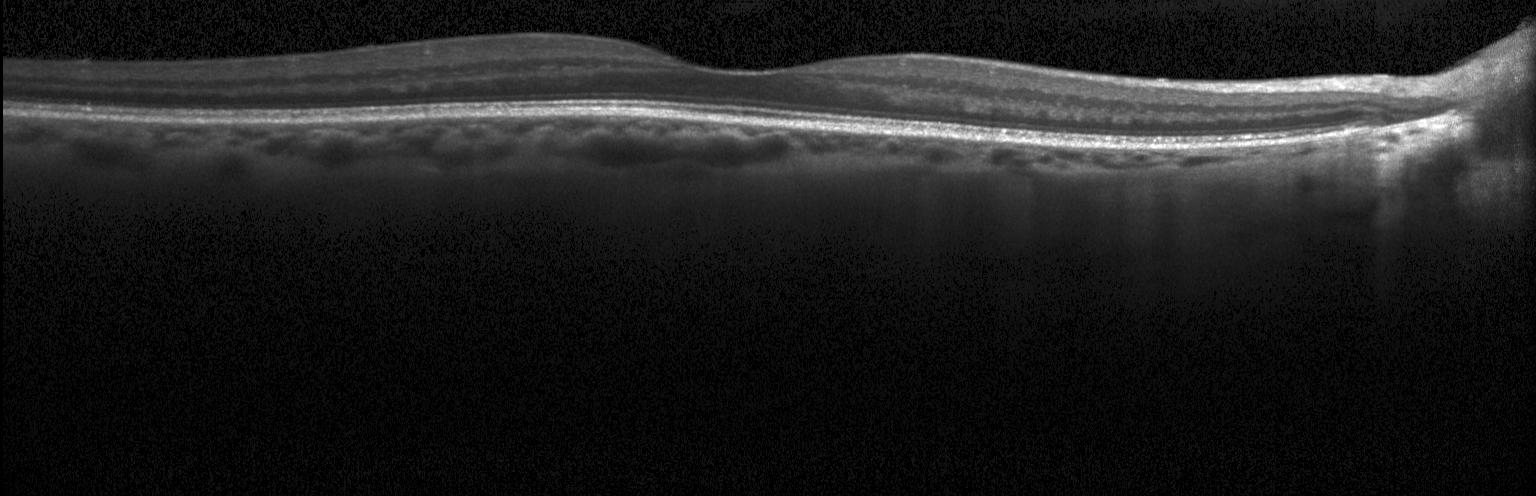

OCT B-scan. Horizontal scan through the fovea.
Diagnosis: no CNV, no DME, and no drusen.